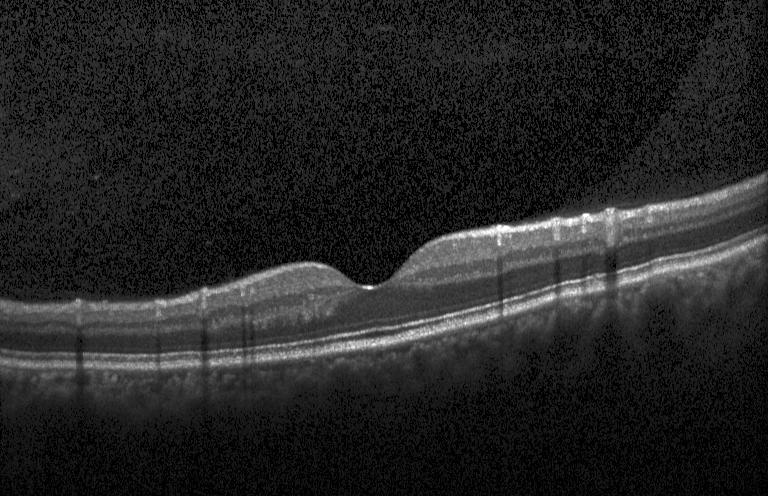
Instrument: Heidelberg Spectralis. Retinal OCT B-scan. Fovea-centered — OCT finding: neither CNV, DME, nor drusen.